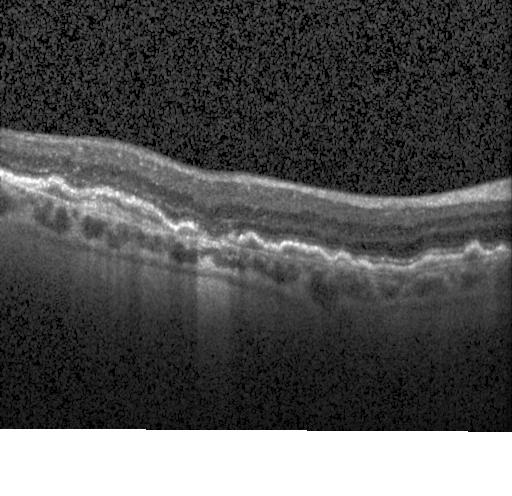 SD-OCT. Retinal OCT cross-section
A choroidal neovascular membrane.